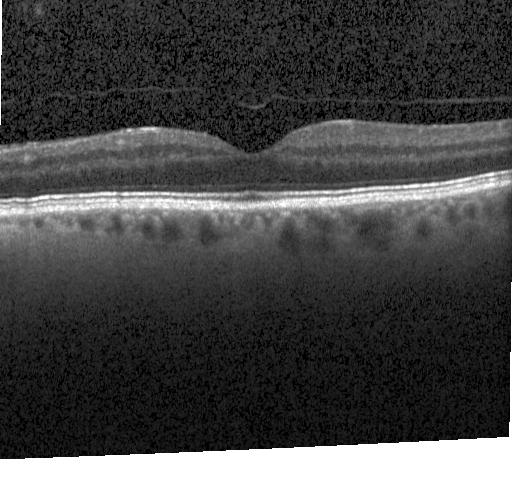
OCT B-scan. The scan shows no evidence of choroidal neovascularization, diabetic macular edema, or drusen.